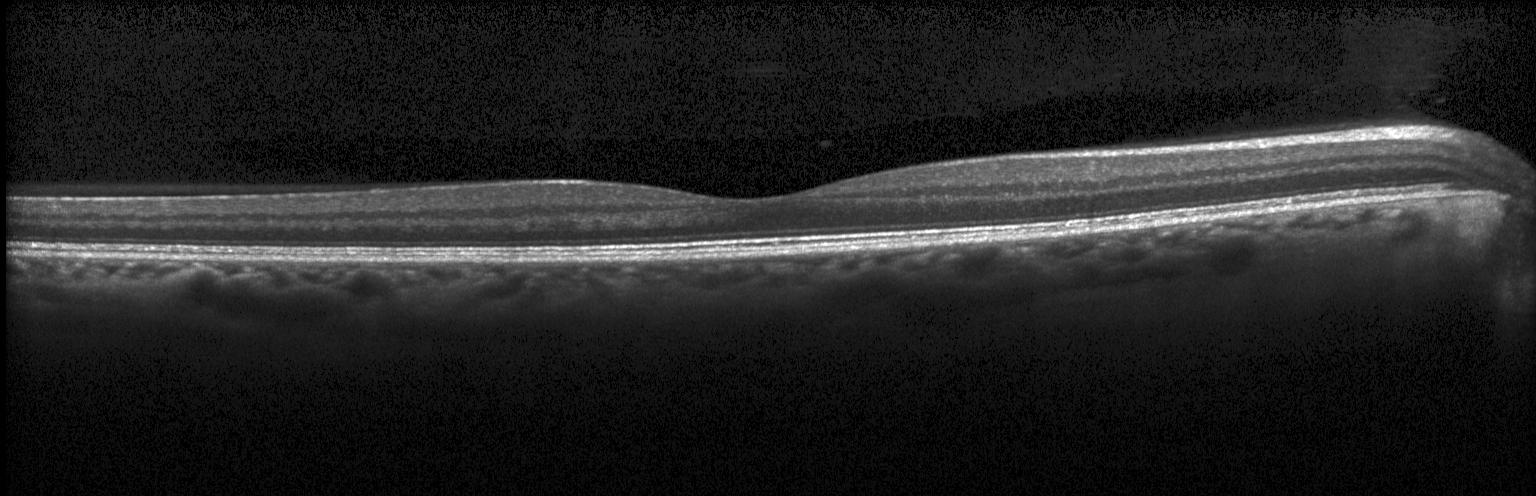

Optical coherence tomography scan · Heidelberg Spectralis OCT system — Impression: no evidence of choroidal neovascularization, diabetic macular edema, or drusen.